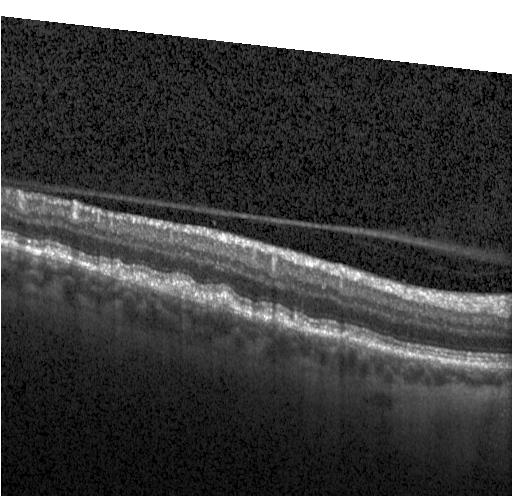 OCT B-scan, acquired on a Heidelberg Spectralis, spectral-domain OCT, centered on the fovea.
Dx: drusen.